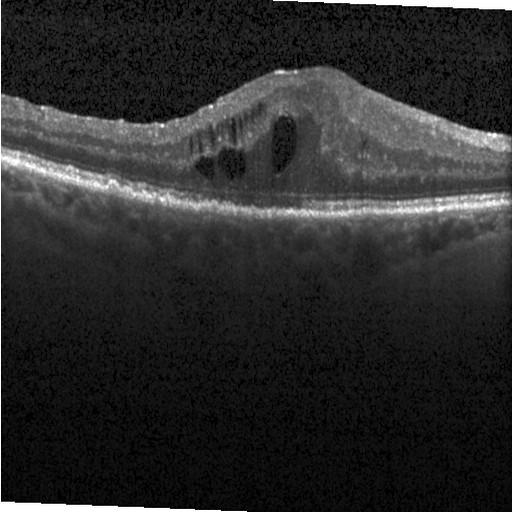

Centered on the fovea; retinal OCT B-scan.
Diabetic macular edema (DME).